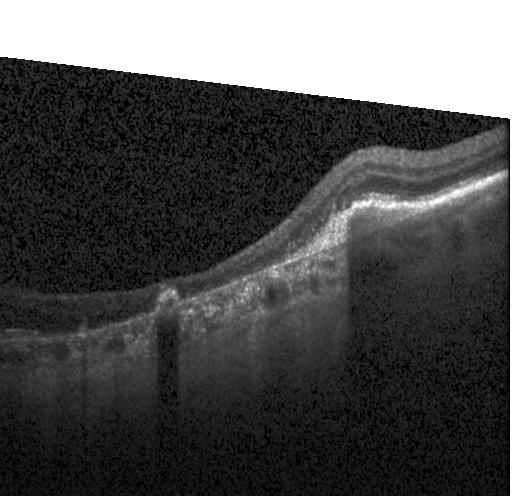
Optical coherence tomography scan · SD-OCT · Heidelberg Spectralis OCT system · centered on the fovea — Finding: choroidal neovascularization.